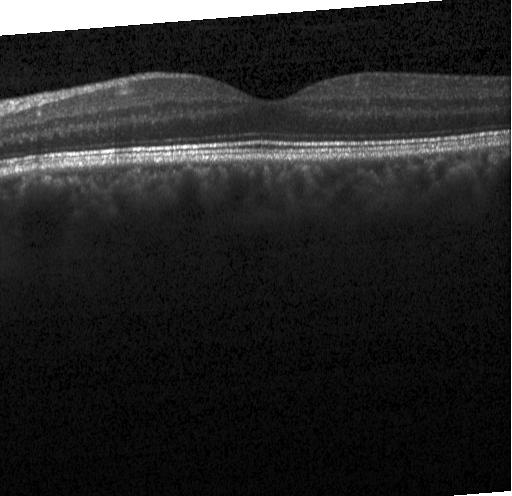
Retinal OCT cross-section — Diagnosis: no choroidal neovascularization, diabetic macular edema, or drusen.